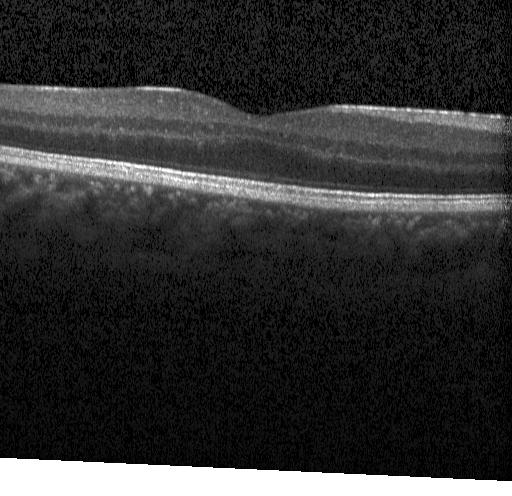

Optical coherence tomography scan — Finding: no evidence of CNV, DME, or drusen.